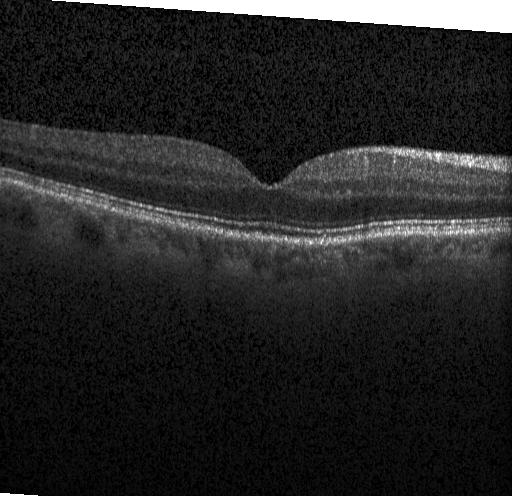

Acquired on a Heidelberg Spectralis · optical coherence tomography B-scan · SD-OCT · through the macula. Diagnosis: neither choroidal neovascularization, diabetic macular edema, nor drusen.